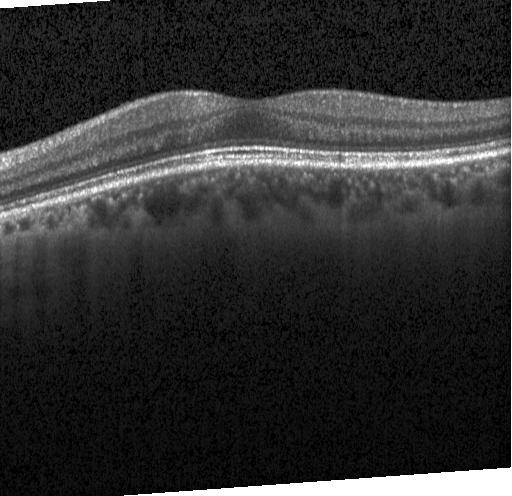

OCT line scan; horizontal scan through the fovea. Assessment: neither CNV, DME, nor drusen.